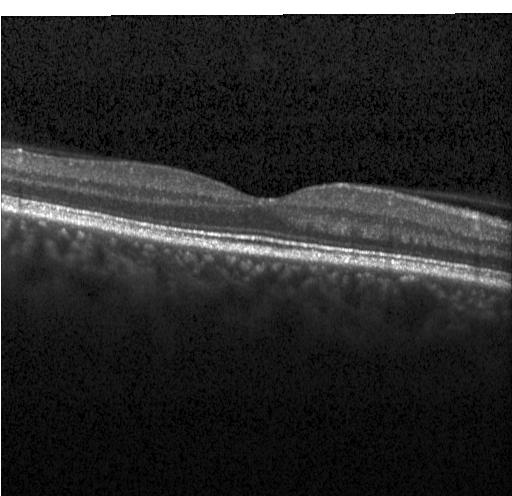
OCT B-scan showing no choroidal neovascularization, no diabetic macular edema, and no drusen.